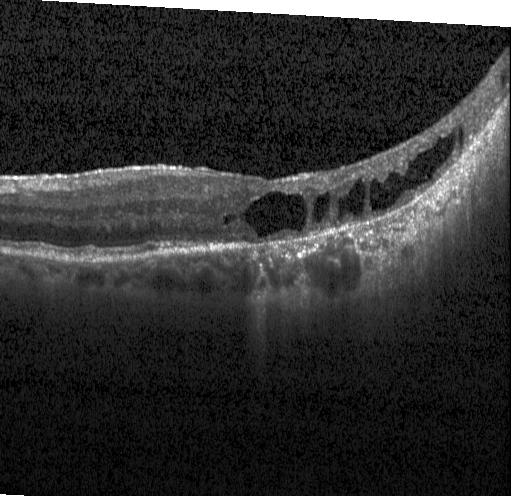
OCT line scan.
Finding: diabetic macular edema.